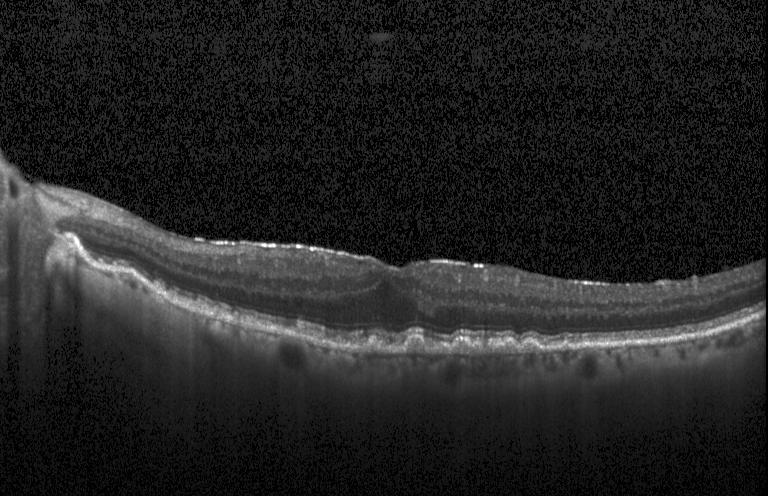
Optical coherence tomography B-scan, spectral-domain optical coherence tomography, instrument: Heidelberg Spectralis
Diagnosis: multiple drusen.